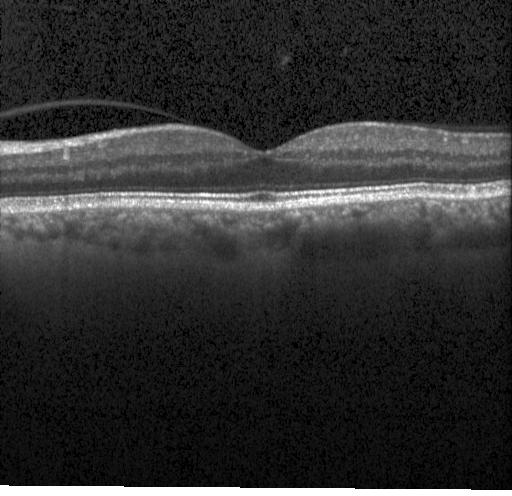

Spectral-domain OCT B-scan: no evidence of choroidal neovascularization, diabetic macular edema, or drusen.